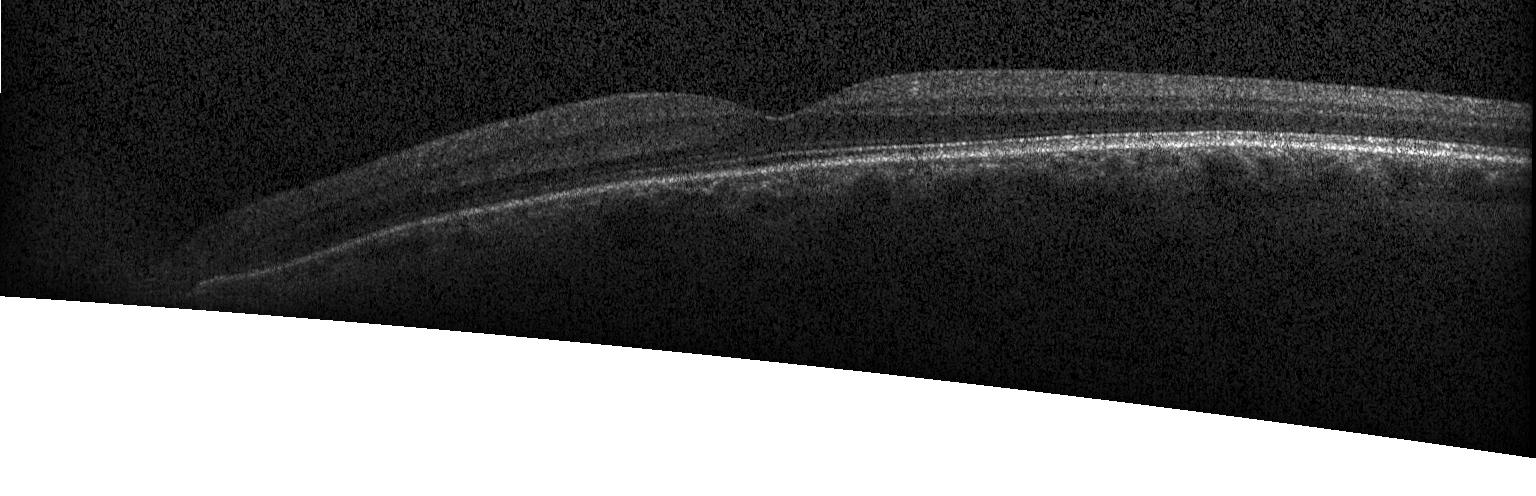

Spectral-domain OCT B-scan: no evidence of CNV, DME, or drusen.